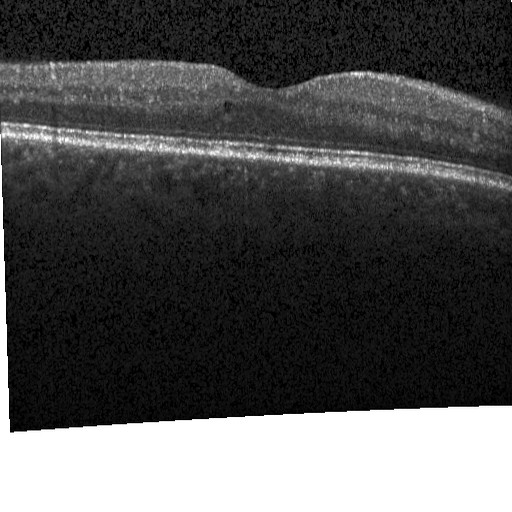

Acquired on a Heidelberg Spectralis; spectral-domain OCT; centered on the fovea; optical coherence tomography B-scan — Impression: diabetic macular edema (DME).